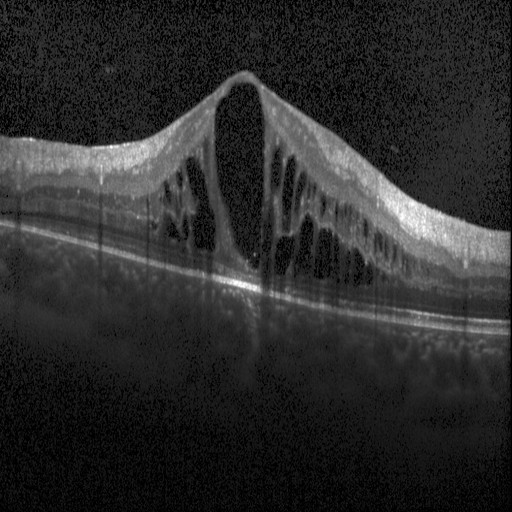 This B-scan demonstrates diabetic macular edema (DME).